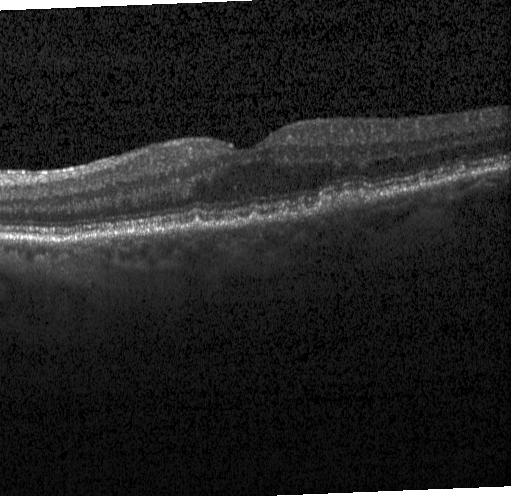
Impression: multiple drusen.